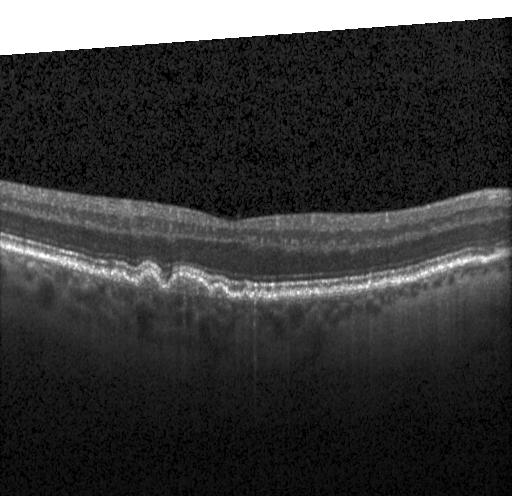

OCT B-scan · spectral-domain optical coherence tomography · Heidelberg Spectralis · horizontal scan through the fovea
Dx: multiple drusen.